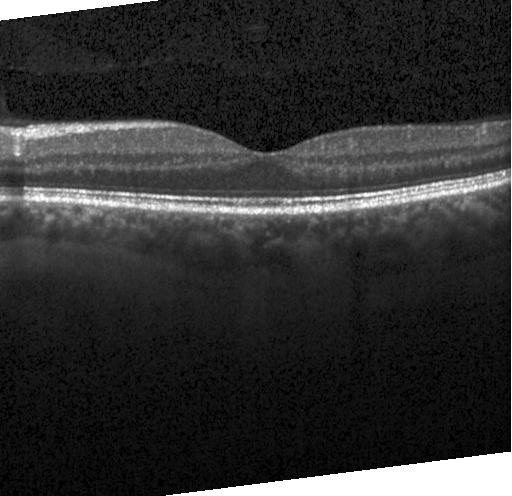 Assessment: no evidence of choroidal neovascularization, diabetic macular edema, or drusen.